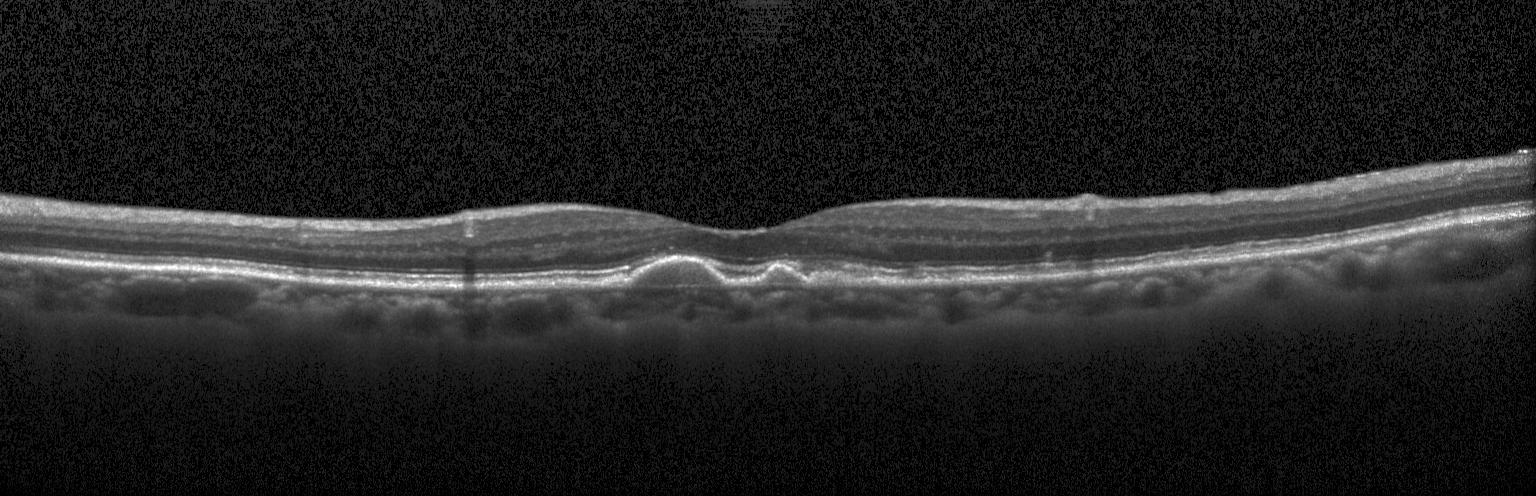

Finding: drusen.